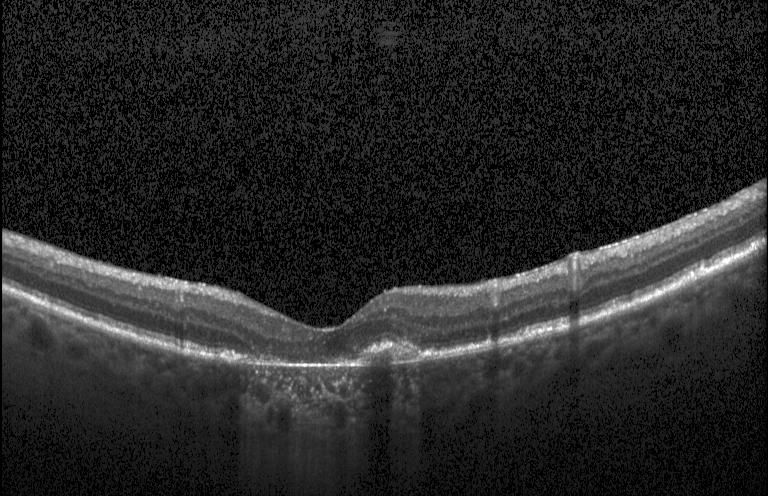
Instrument: Heidelberg Spectralis; retinal OCT cross-section; centered on the fovea.
This B-scan demonstrates choroidal neovascularization.